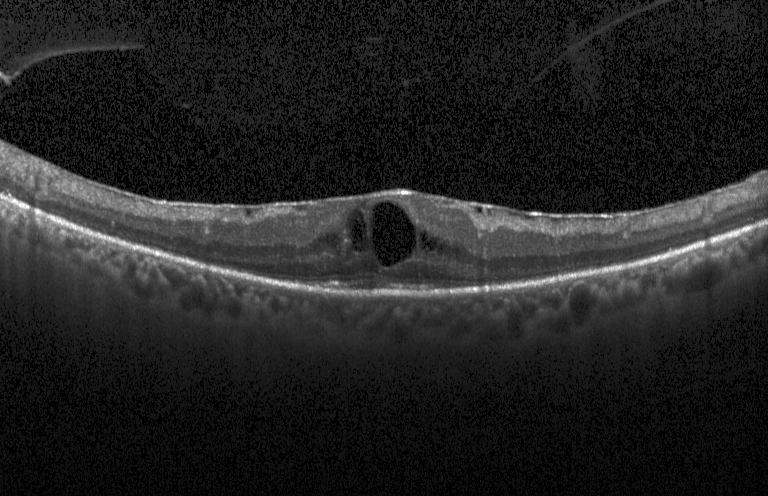
Spectral-domain OCT B-scan: DME.